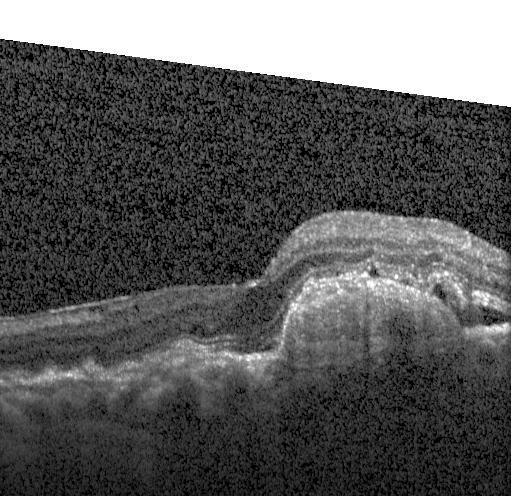

The scan shows a choroidal neovascular membrane.